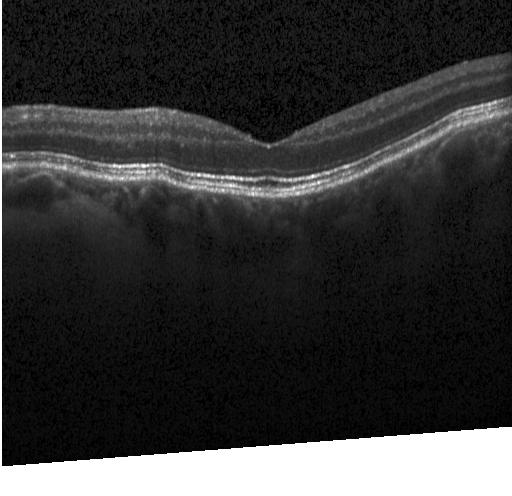 Finding: no CNV, no DME, and no drusen.